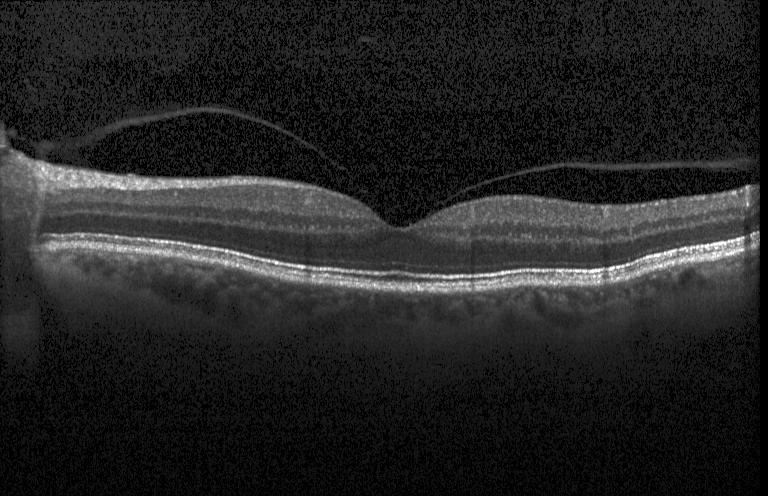 OCT line scan. Heidelberg Spectralis
Macular OCT: no CNV, no DME, and no drusen.